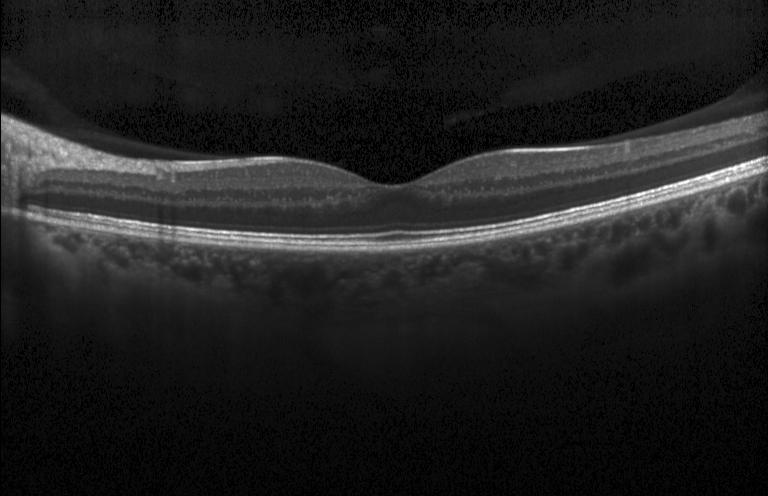 Retinal OCT B-scan, horizontal scan through the fovea, Heidelberg Spectralis, spectral-domain optical coherence tomography
Assessment: neither CNV, DME, nor drusen.